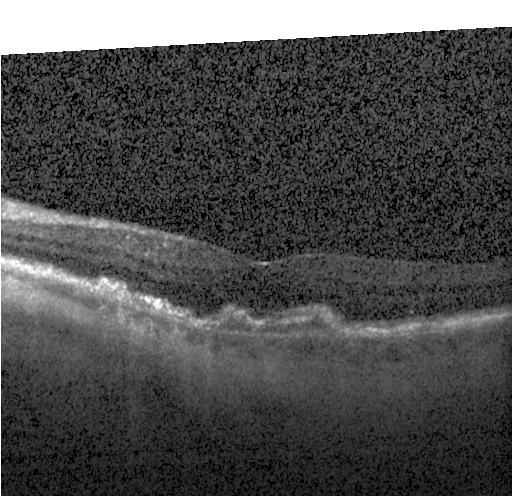

Spectral-domain optical coherence tomography, OCT line scan.
Macular OCT: a choroidal neovascular membrane.